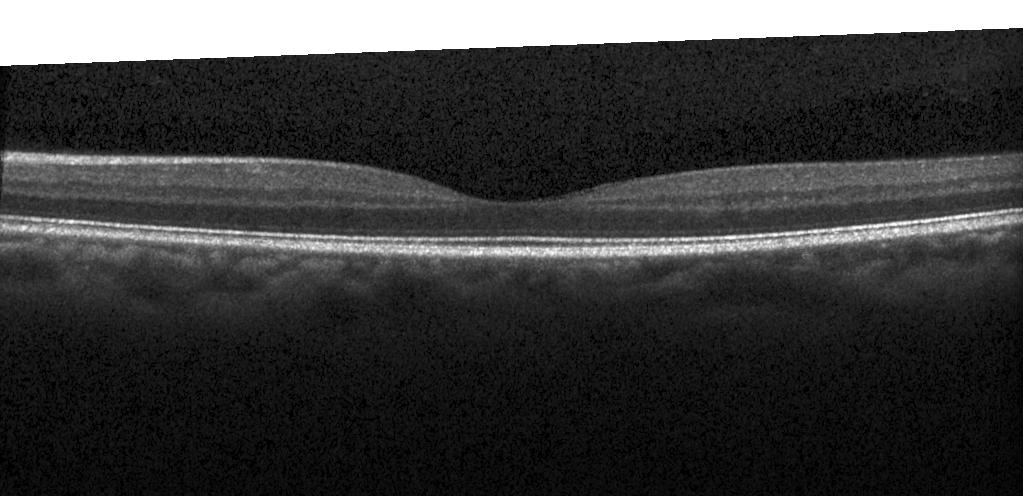
Diagnosis: neither choroidal neovascularization, diabetic macular edema, nor drusen.